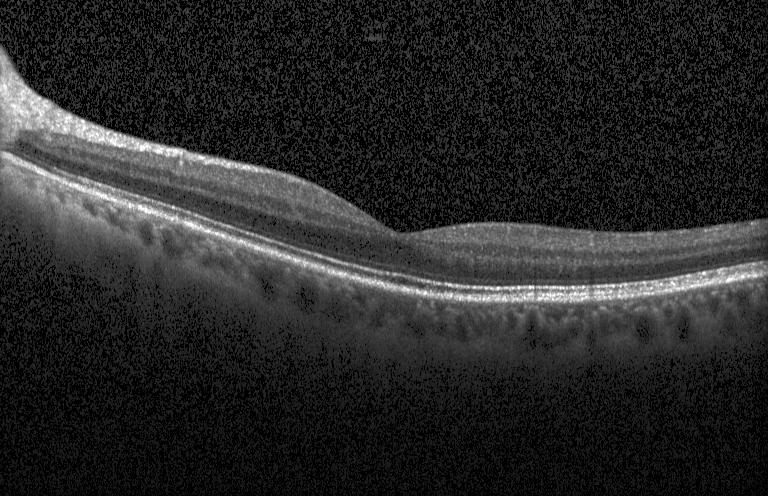 Diagnosis: no choroidal neovascularization, no diabetic macular edema, and no drusen.